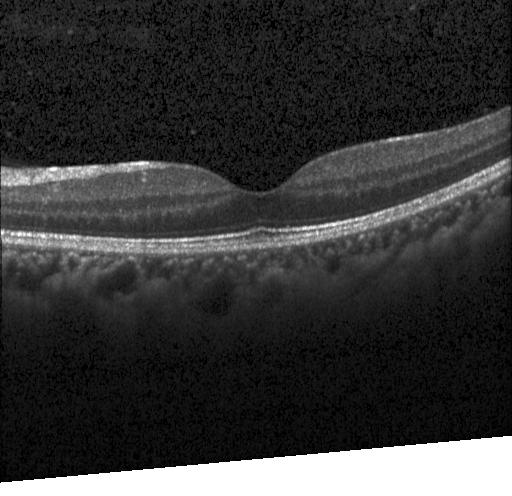

OCT B-scan — Diagnosis: neither choroidal neovascularization, diabetic macular edema, nor drusen.